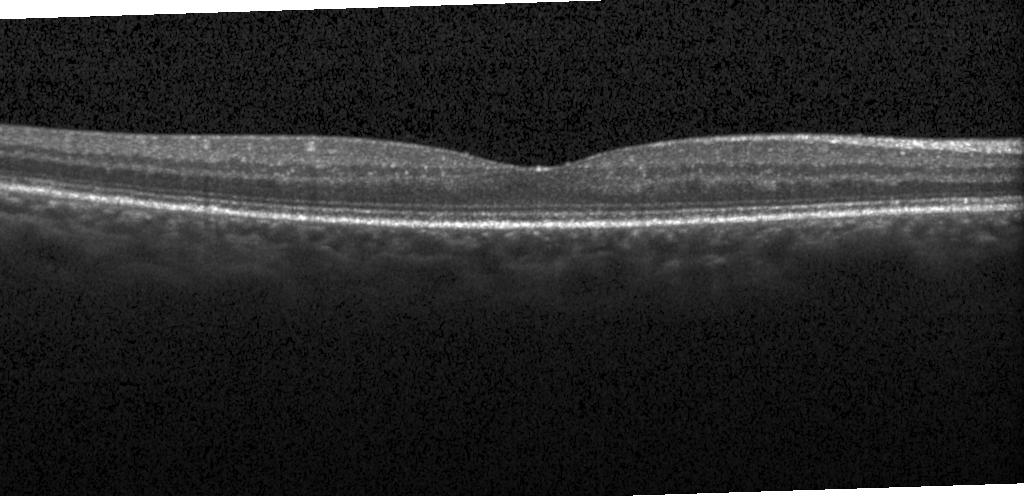 Heidelberg Spectralis OCT system · spectral-domain OCT · retinal OCT B-scan · through the macula.
This B-scan demonstrates no choroidal neovascularization, no diabetic macular edema, and no drusen.